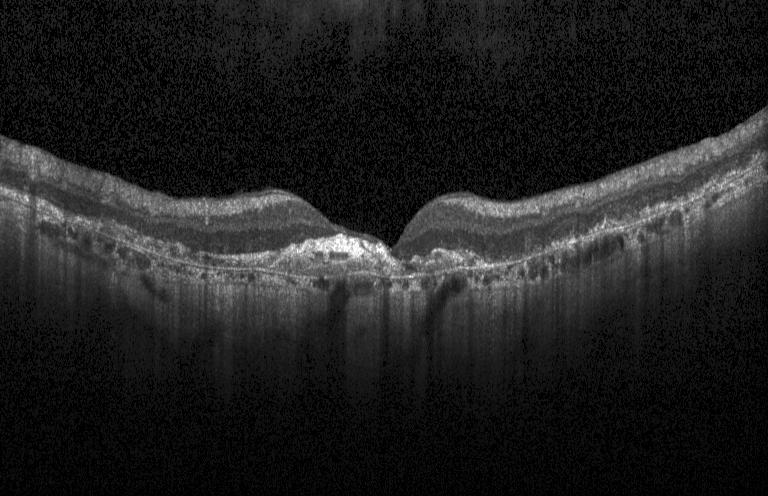
Spectral-domain optical coherence tomography, optical coherence tomography B-scan, horizontal scan through the fovea, acquired on a Heidelberg Spectralis — Assessment: a choroidal neovascular membrane.